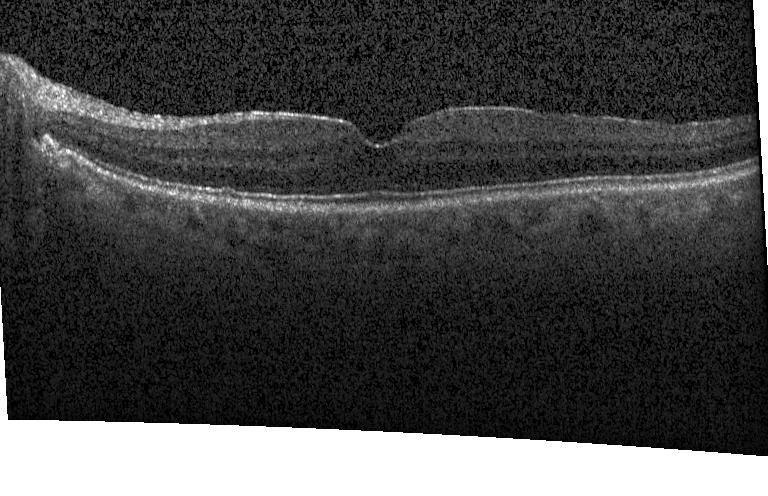 Impression: no choroidal neovascularization, no diabetic macular edema, and no drusen.